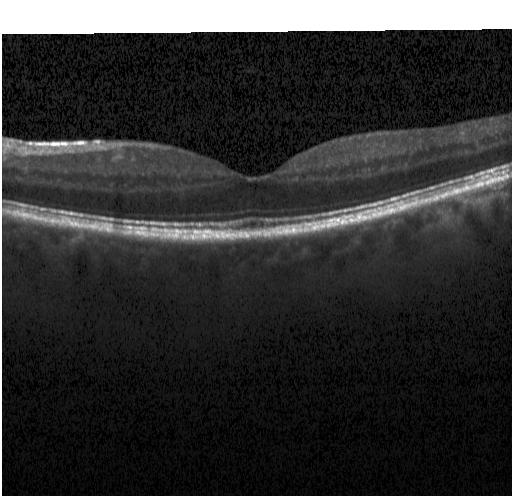

Heidelberg Spectralis OCT system · OCT B-scan · spectral-domain OCT · centered on the fovea
No choroidal neovascularization, diabetic macular edema, or drusen.